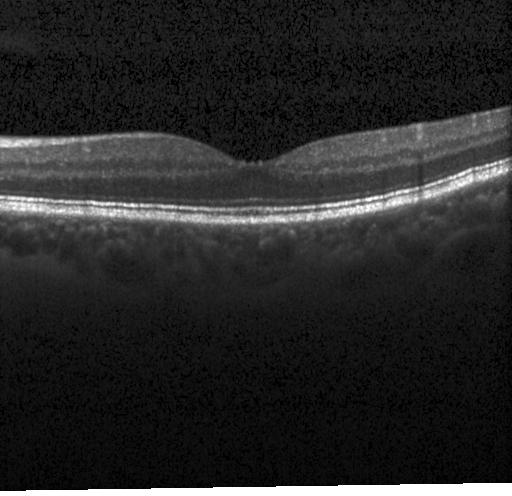 OCT B-scan.
Diagnosis: no choroidal neovascularization, diabetic macular edema, or drusen.